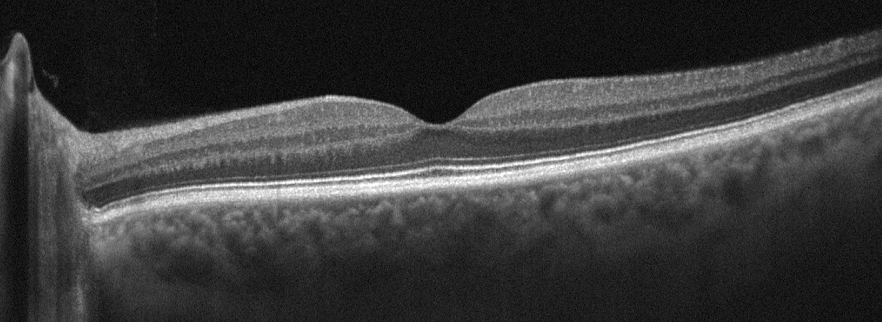
Left eye; acquired on an Optovue Avanti RTVue XR; OCT B-scan.
Impression: no evidence of AMD, DME, ERM, RAO, RVO, or VID.